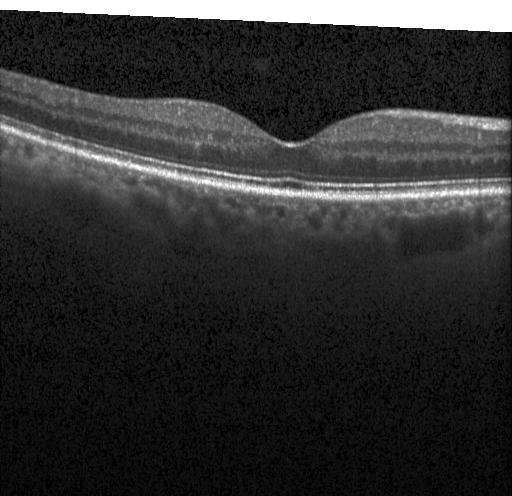
Retinal OCT cross-section showing no evidence of choroidal neovascularization, diabetic macular edema, or drusen.